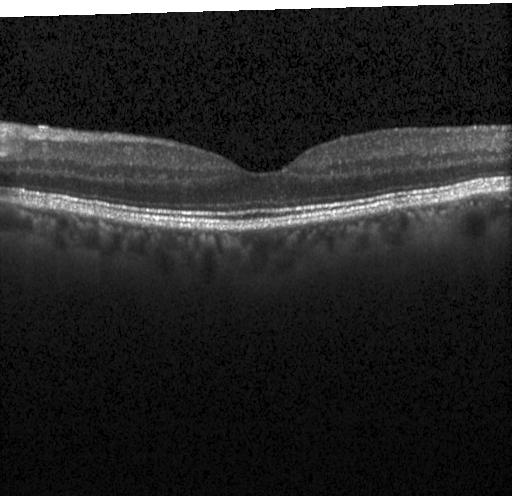 OCT B-scan. SD-OCT — Finding: neither choroidal neovascularization, diabetic macular edema, nor drusen.